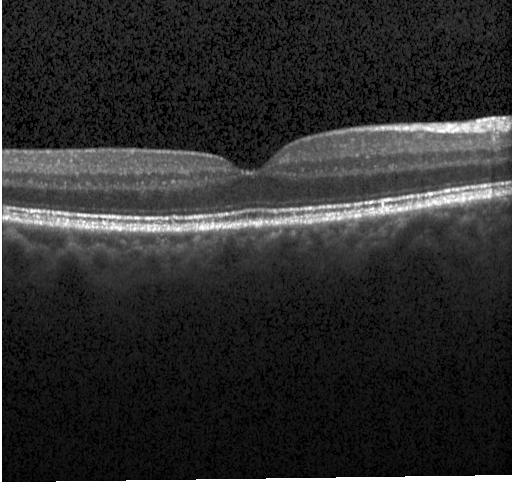

The scan shows no choroidal neovascularization, diabetic macular edema, or drusen.